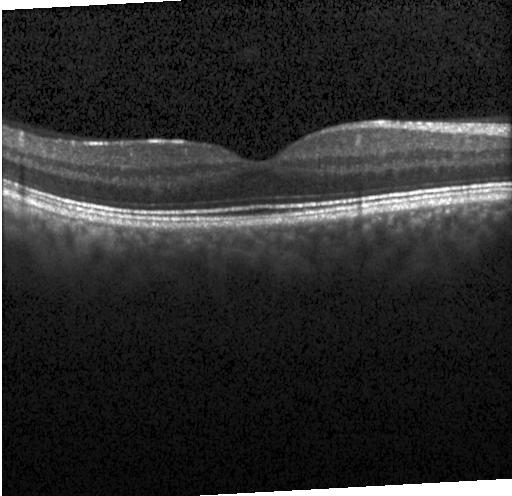

OCT B-scan — Assessment: no evidence of choroidal neovascularization, diabetic macular edema, or drusen.